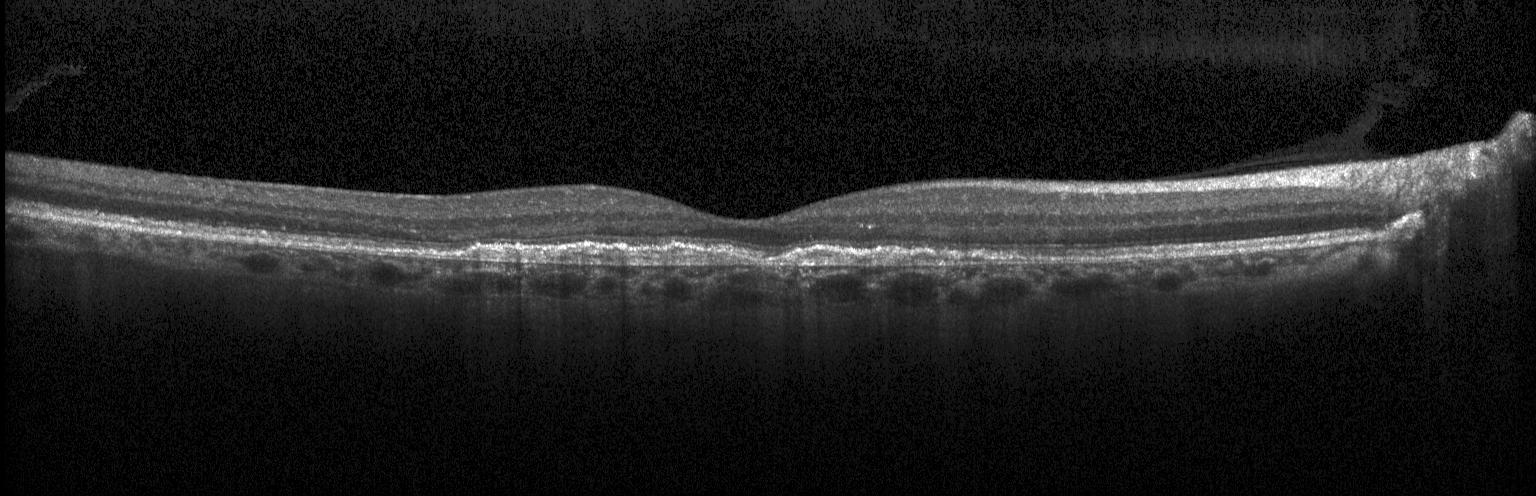
Spectral-domain OCT B-scan: no choroidal neovascularization, no diabetic macular edema, and no drusen.